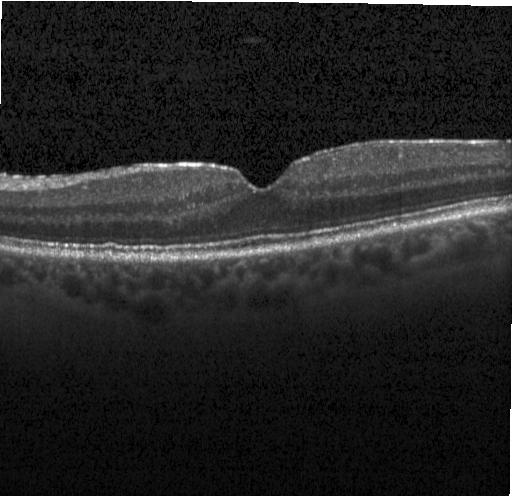
Finding: no evidence of choroidal neovascularization, diabetic macular edema, or drusen.